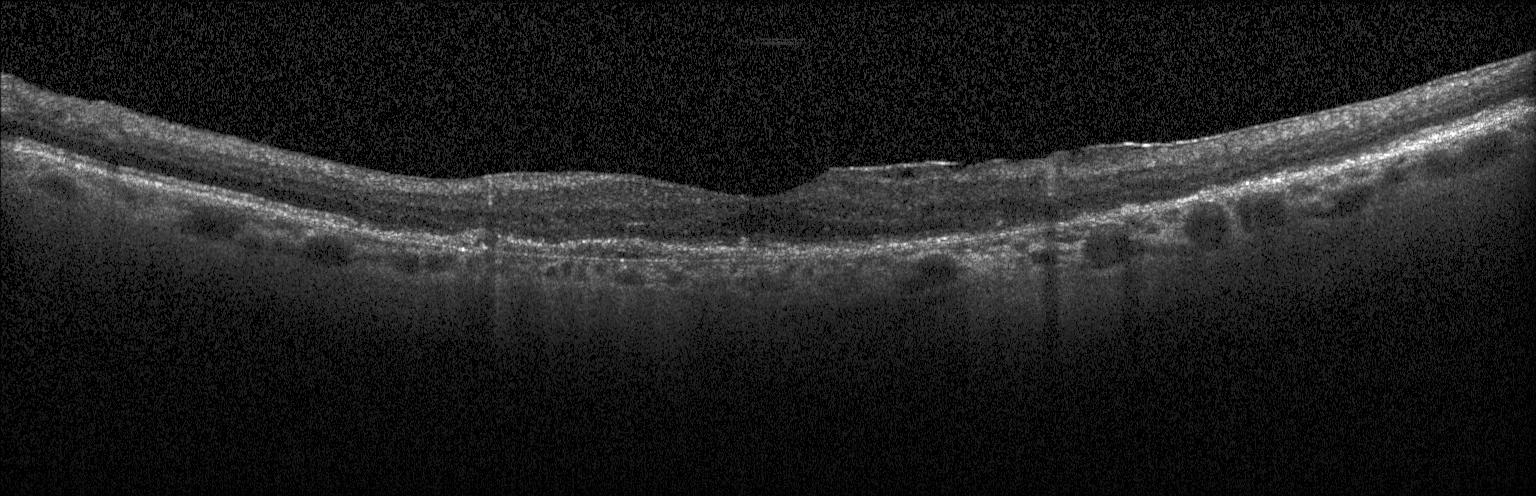 Through the macula; optical coherence tomography B-scan; instrument: Heidelberg Spectralis.
OCT finding: choroidal neovascularization (CNV).